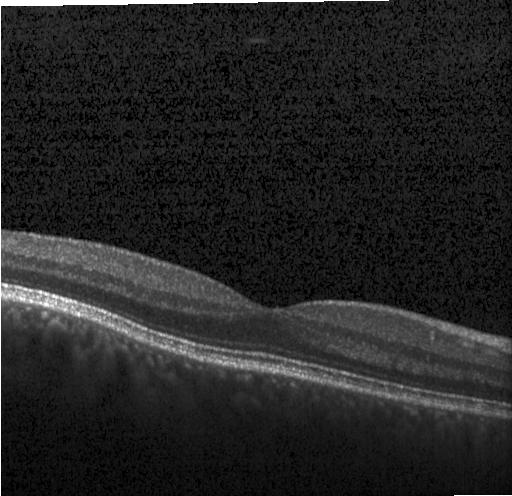

Retinal OCT cross-section, SD-OCT, fovea-centered, Heidelberg Spectralis OCT system.
Impression: neither CNV, DME, nor drusen.